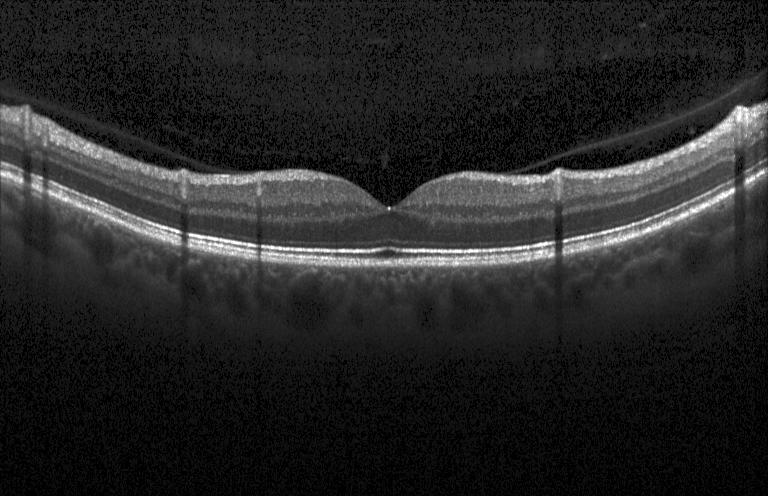

Diagnosis: no evidence of choroidal neovascularization, diabetic macular edema, or drusen.